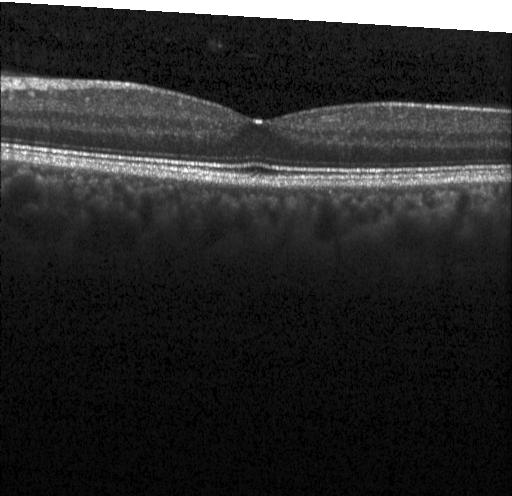
Macular scan. SD-OCT. Retinal OCT cross-section. Instrument: Heidelberg Spectralis. Assessment: no choroidal neovascularization, diabetic macular edema, or drusen.